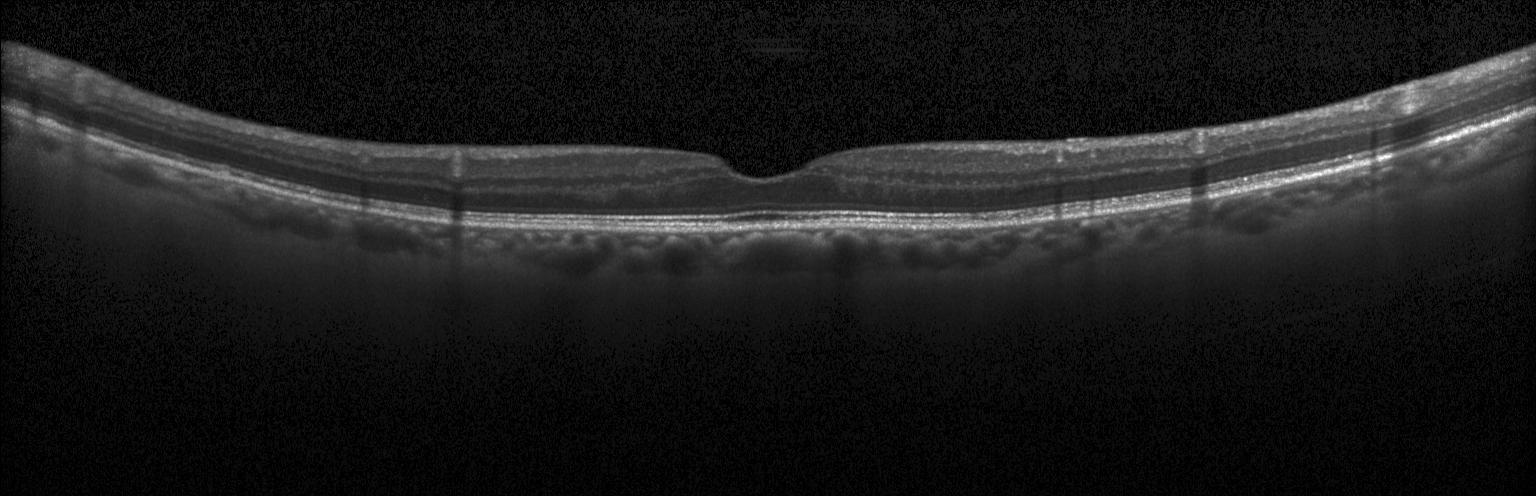

Finding: no evidence of CNV, DME, or drusen.